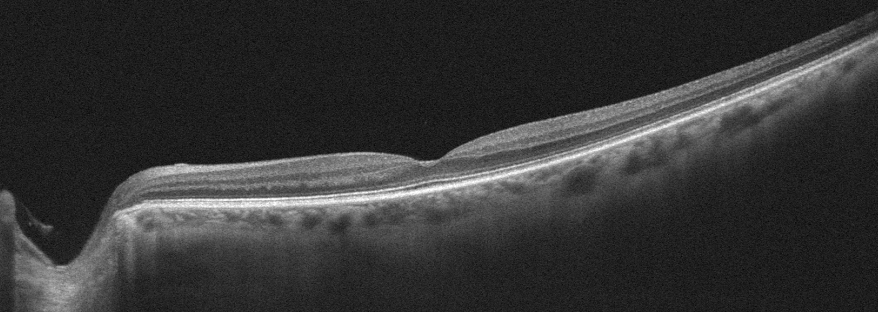 Dx: no AMD, DME, ERM, RAO, RVO, or VID.